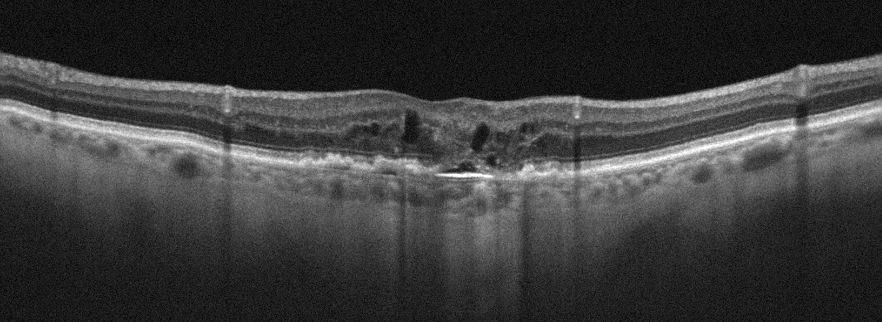

Oculus dexter; optical coherence tomography scan; macular scan.
Finding: AMD.